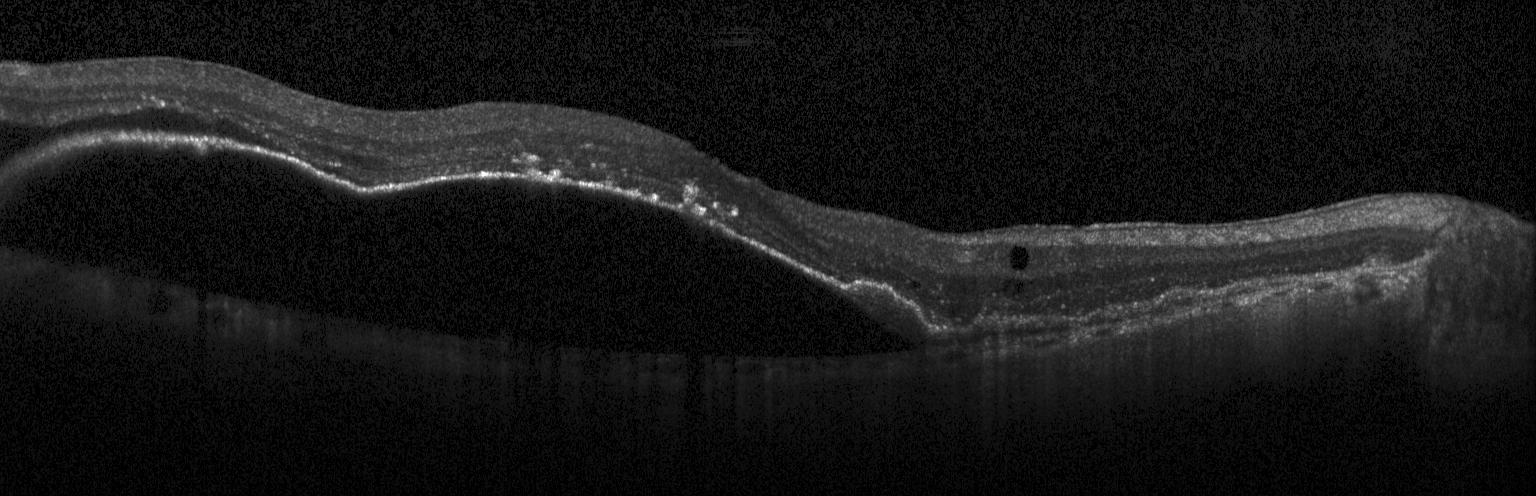 Instrument: Heidelberg Spectralis, centered on the fovea, OCT line scan
This B-scan demonstrates choroidal neovascularization.